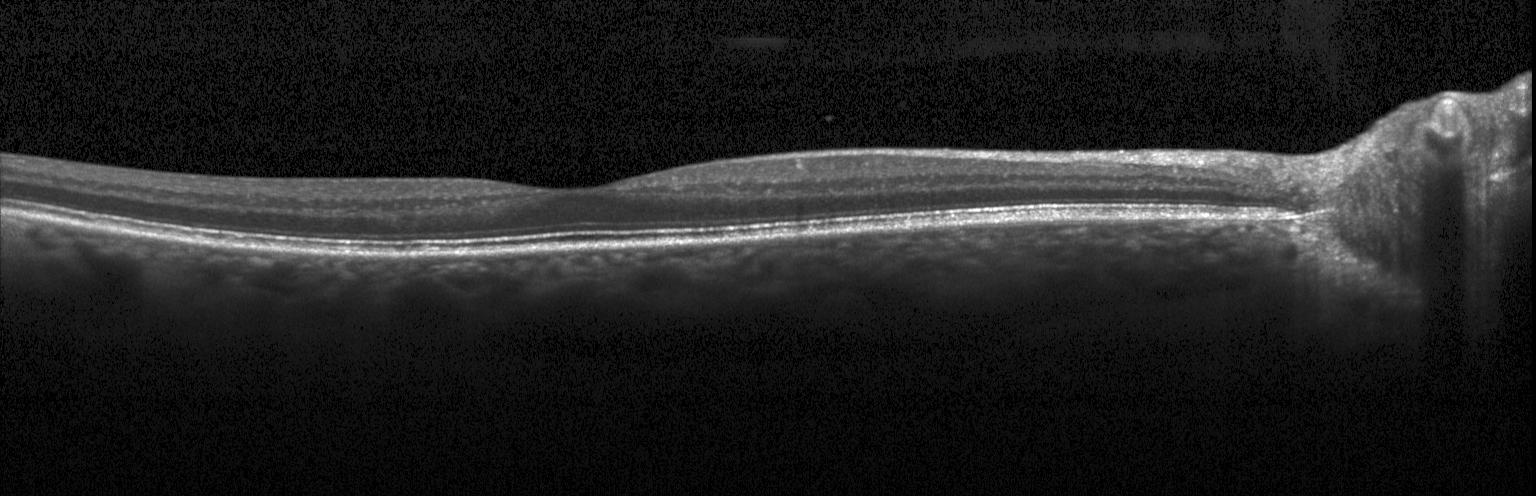

Instrument: Heidelberg Spectralis, optical coherence tomography scan, spectral-domain OCT — Diagnosis: no evidence of CNV, DME, or drusen.